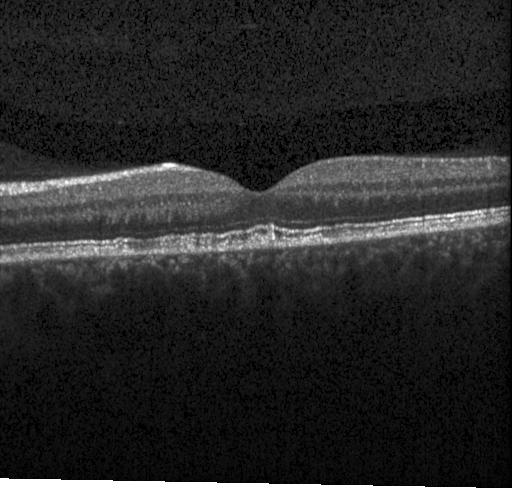 Macular OCT: multiple drusen.